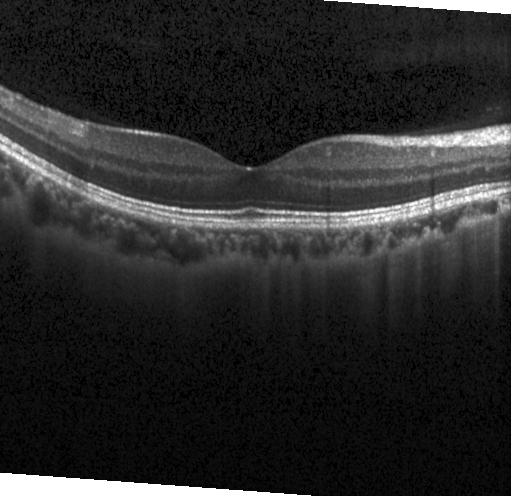
Optical coherence tomography scan; instrument: Heidelberg Spectralis; fovea-centered
Macular OCT: neither CNV, DME, nor drusen.